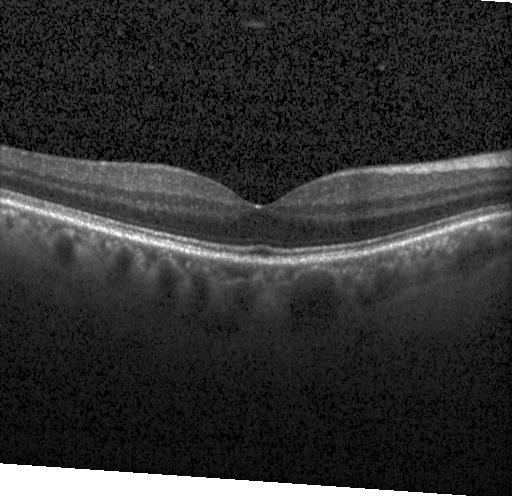

Heidelberg Spectralis; horizontal scan through the fovea; optical coherence tomography scan; spectral-domain optical coherence tomography.
The scan shows no choroidal neovascularization, diabetic macular edema, or drusen.